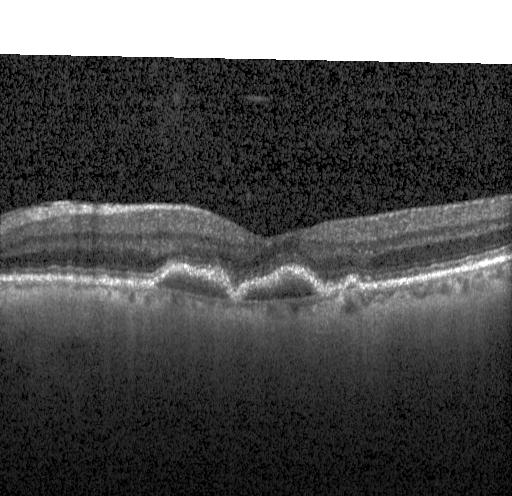 Impression: choroidal neovascularization.